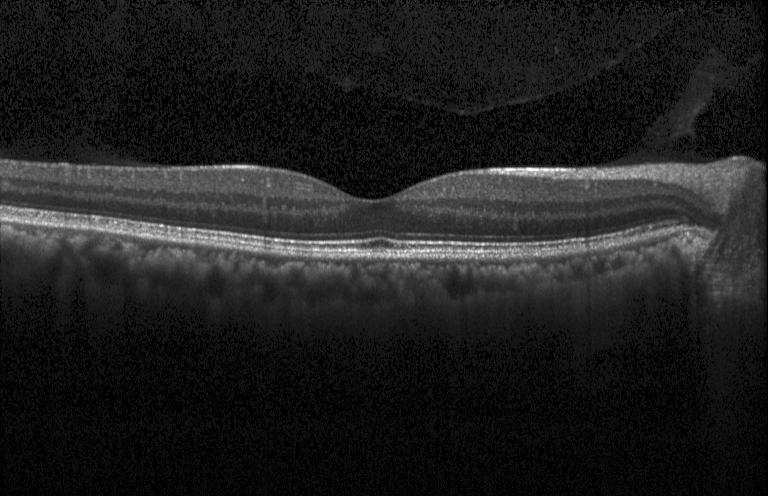 OCT B-scan. Macular OCT: no CNV, no DME, and no drusen.